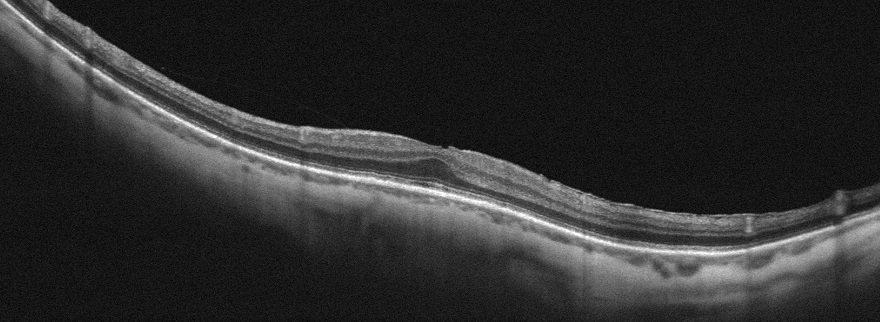
OCT B-scan. Instrument: Optovue Avanti RTVue XR. Macular scan. Assessment: epiretinal membrane (ERM).